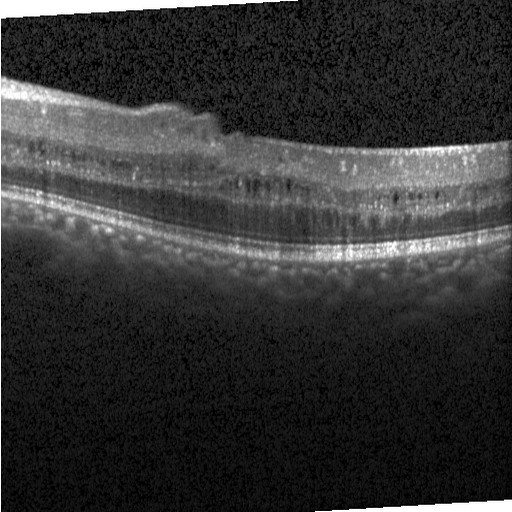
Retinal OCT B-scan, instrument: Heidelberg Spectralis. Diagnosis: DME.